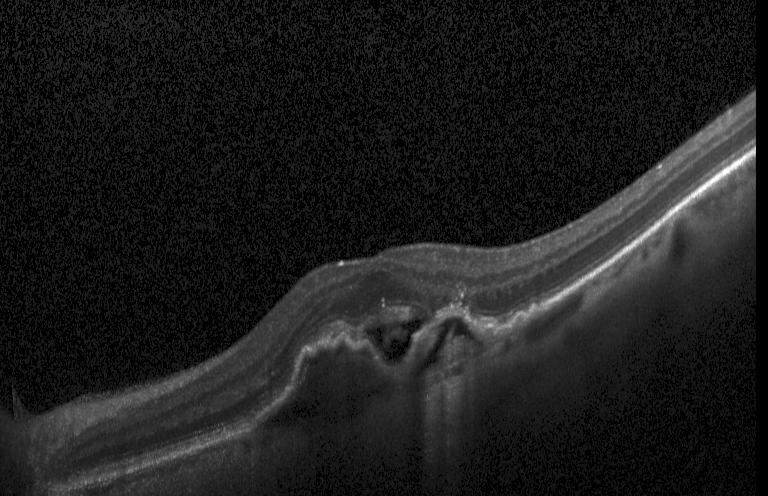
Macular scan; OCT line scan.
OCT finding: choroidal neovascularization (CNV).